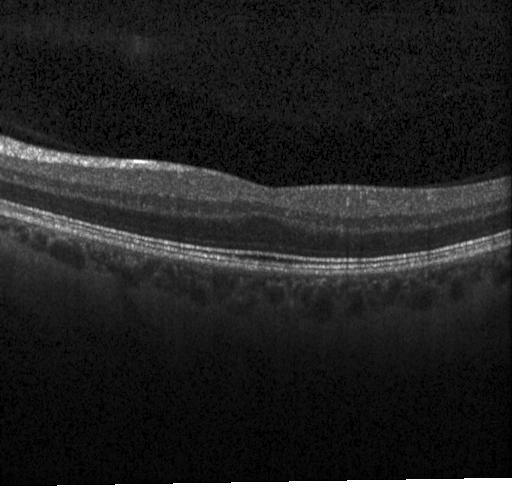
Macular OCT: no choroidal neovascularization, diabetic macular edema, or drusen.